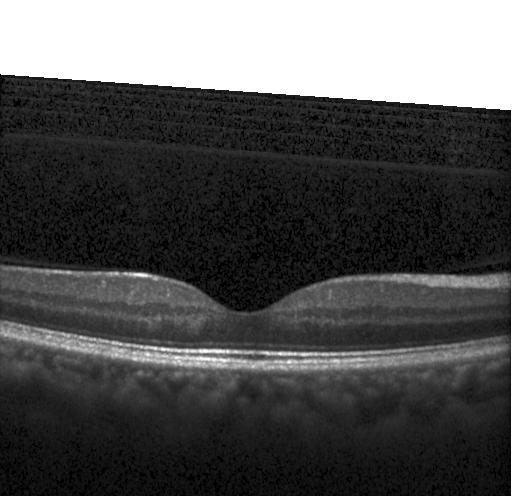
Retinal OCT B-scan; macular scan
Assessment: neither choroidal neovascularization, diabetic macular edema, nor drusen.